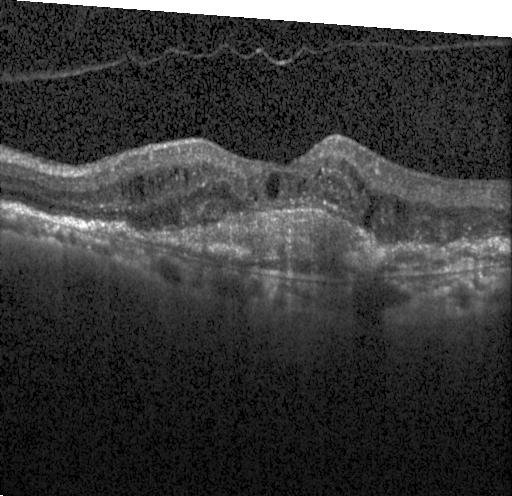

Finding: a choroidal neovascular membrane.